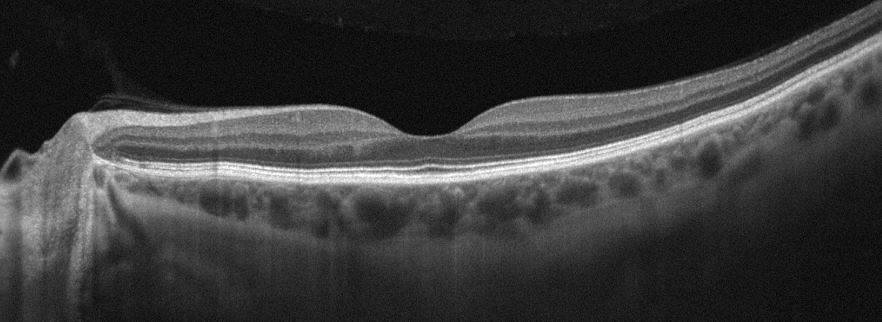

OS · optical coherence tomography scan
Finding: absence of AMD, DME, ERM, RAO, RVO, and vitreomacular interface disease.